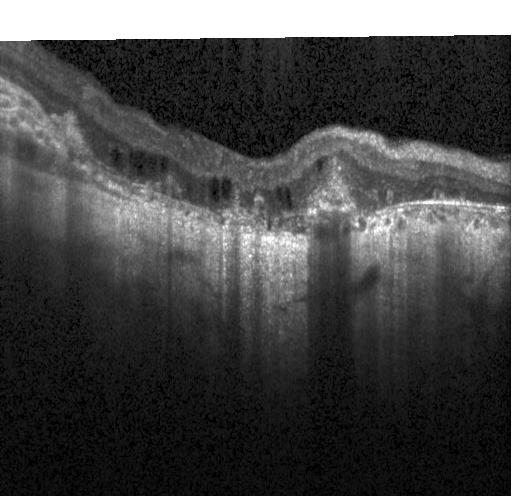
Retinal OCT cross-section. This B-scan demonstrates a choroidal neovascular membrane.